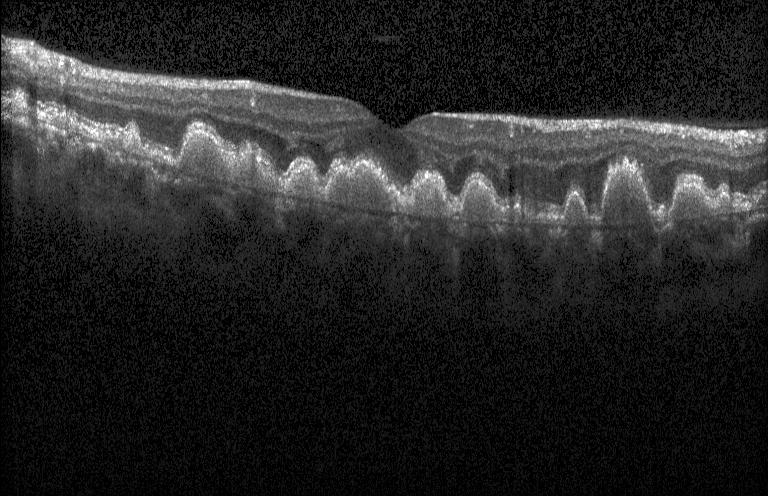 OCT line scan — Assessment: drusen.